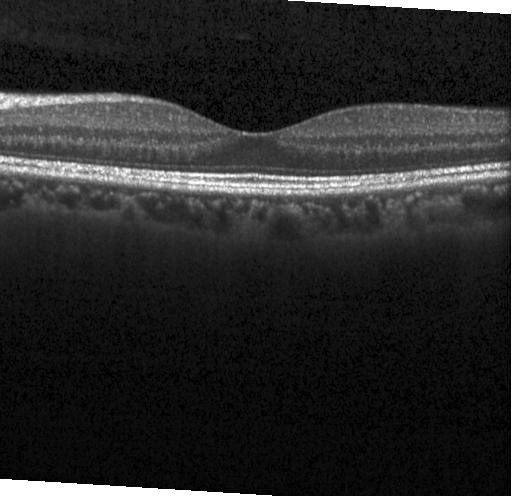 Impression: neither CNV, DME, nor drusen.